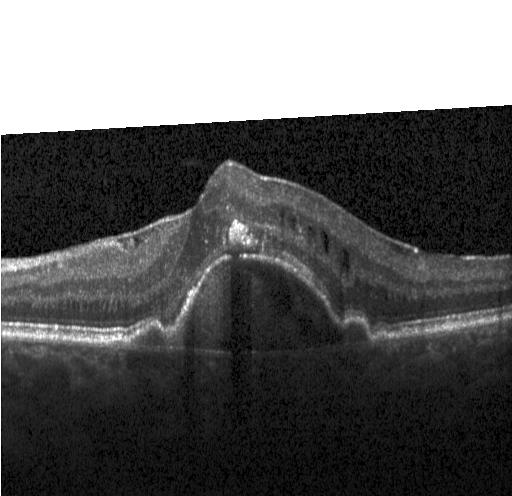
Optical coherence tomography B-scan — The scan shows a choroidal neovascular membrane.